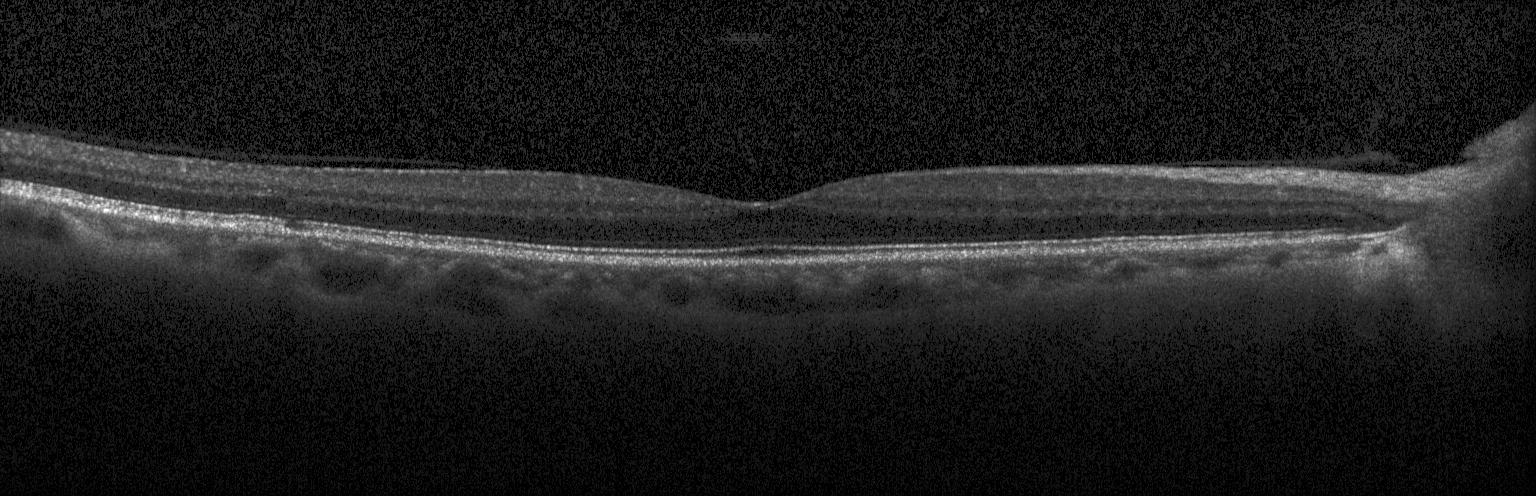

Spectral-domain optical coherence tomography; OCT B-scan
Impression: no evidence of choroidal neovascularization, diabetic macular edema, or drusen.